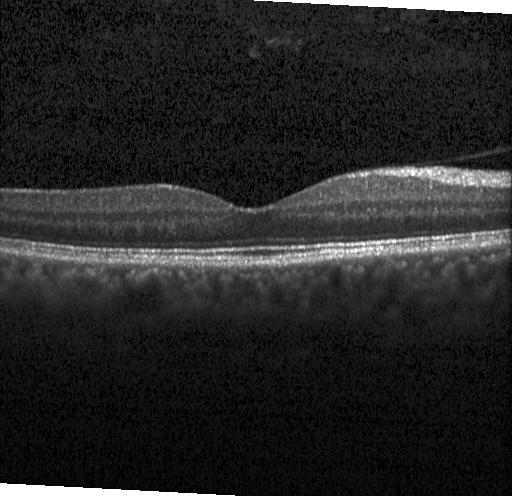 OCT B-scan. Instrument: Heidelberg Spectralis
This B-scan demonstrates no choroidal neovascularization, no diabetic macular edema, and no drusen.